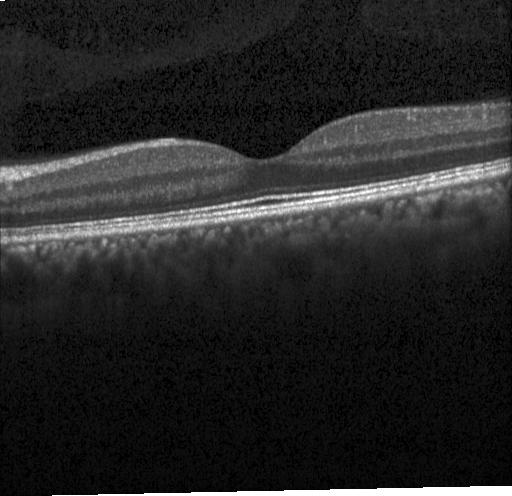
Centered on the fovea; Heidelberg Spectralis OCT system; optical coherence tomography B-scan.
Finding: no evidence of choroidal neovascularization, diabetic macular edema, or drusen.